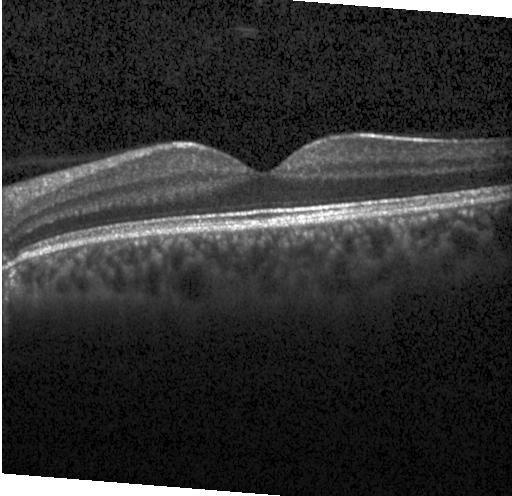 Dx: neither choroidal neovascularization, diabetic macular edema, nor drusen.